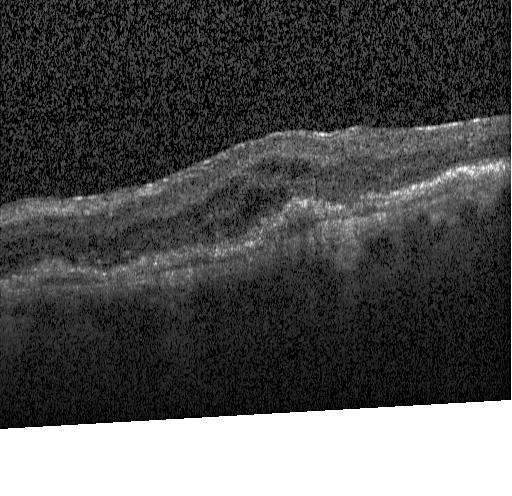
Spectral-domain OCT · OCT B-scan
OCT finding: choroidal neovascularization.